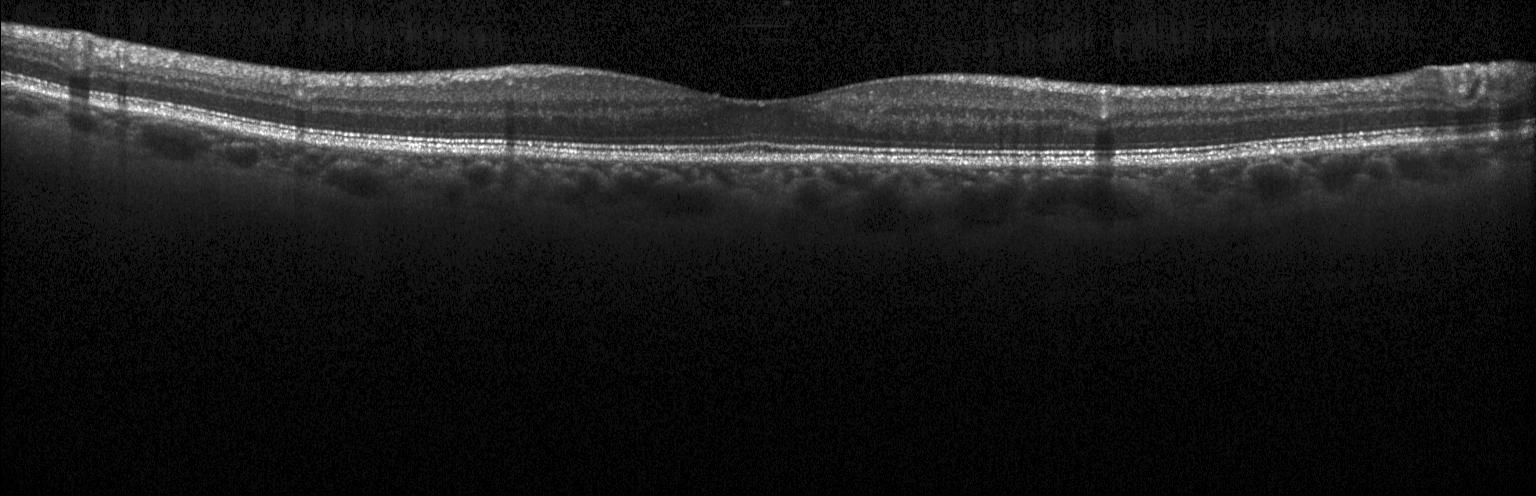

Retinal OCT cross-section; centered on the fovea
The scan shows no choroidal neovascularization, no diabetic macular edema, and no drusen.